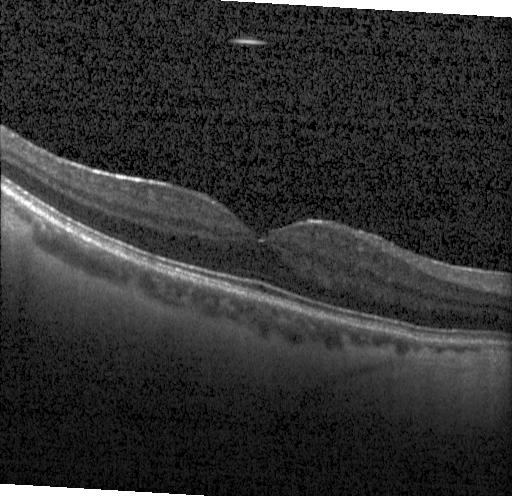

Instrument: Heidelberg Spectralis · optical coherence tomography scan
Impression: no choroidal neovascularization, diabetic macular edema, or drusen.